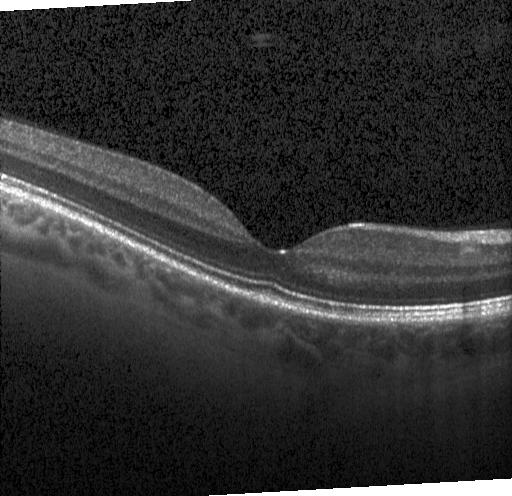
Retinal OCT cross-section — Diagnosis: no evidence of choroidal neovascularization, diabetic macular edema, or drusen.